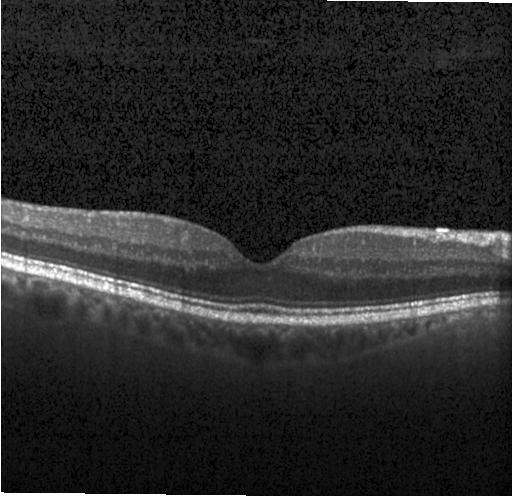
Retinal OCT cross-section, spectral-domain OCT.
Impression: neither CNV, DME, nor drusen.